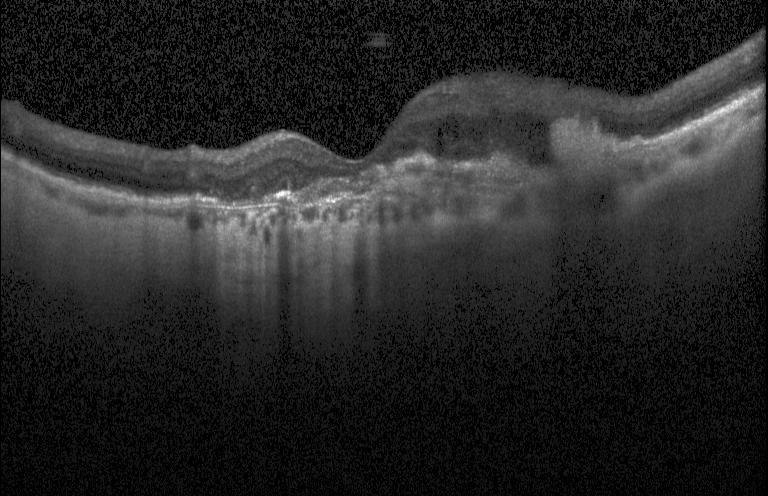
Retinal OCT cross-section — Assessment: choroidal neovascularization.